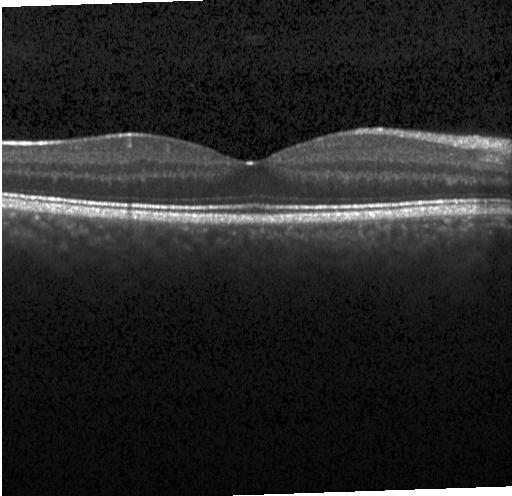

OCT line scan.
Impression: no CNV, DME, or drusen.